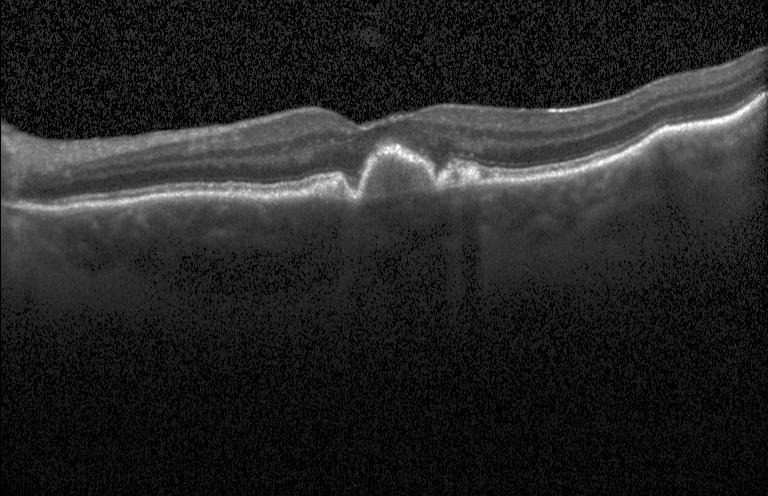

Optical coherence tomography B-scan. Acquired on a Heidelberg Spectralis. Centered on the fovea. The scan shows drusen.